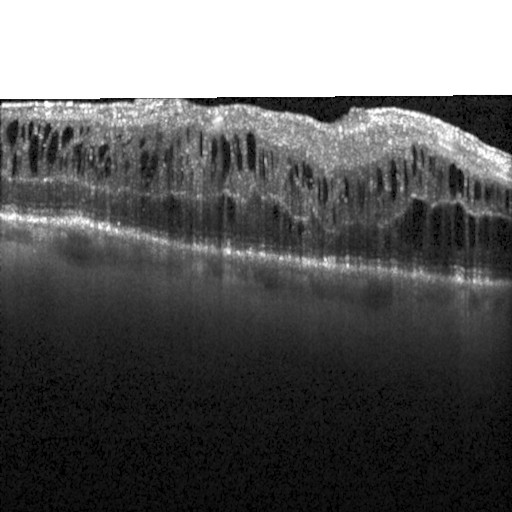

SD-OCT, OCT line scan, Heidelberg Spectralis.
Dx: diabetic macular edema.